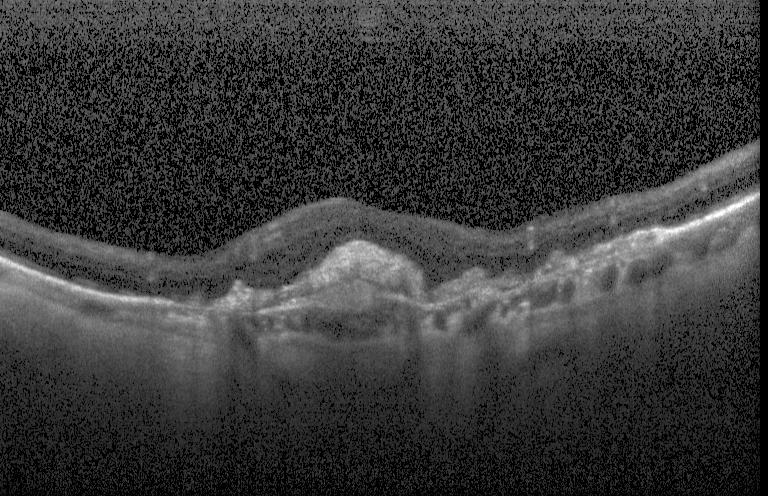 Optical coherence tomography scan
Macular OCT: choroidal neovascularization (CNV).